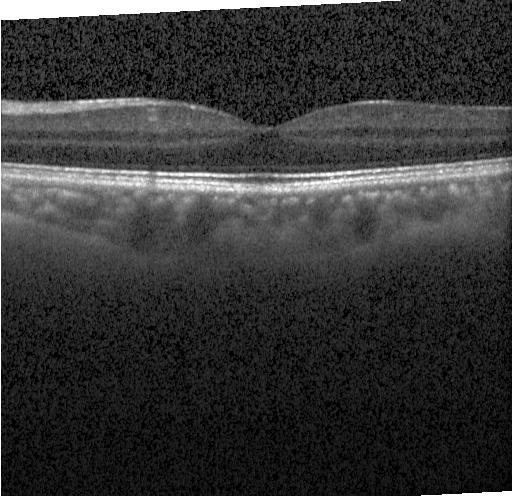 Impression: no choroidal neovascularization, no diabetic macular edema, and no drusen.